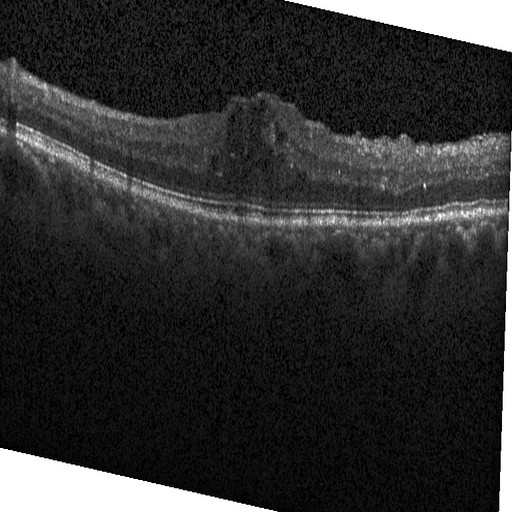
Dx: DME.